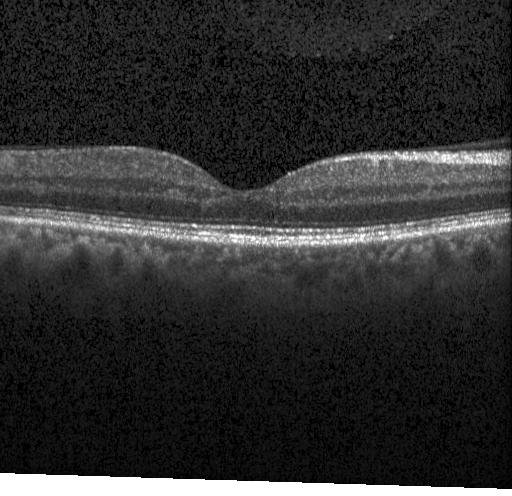

Macular OCT: neither choroidal neovascularization, diabetic macular edema, nor drusen.